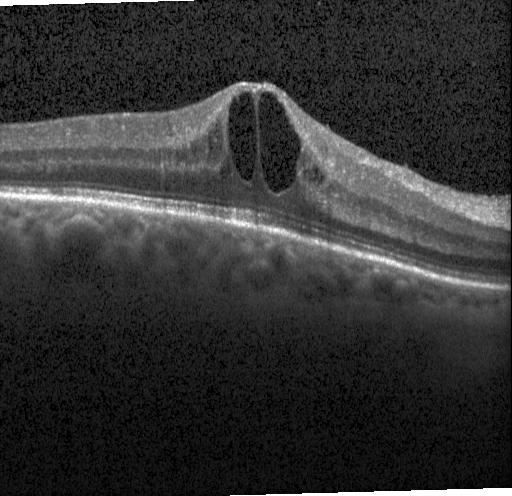 Optical coherence tomography B-scan. The scan shows diabetic macular edema.